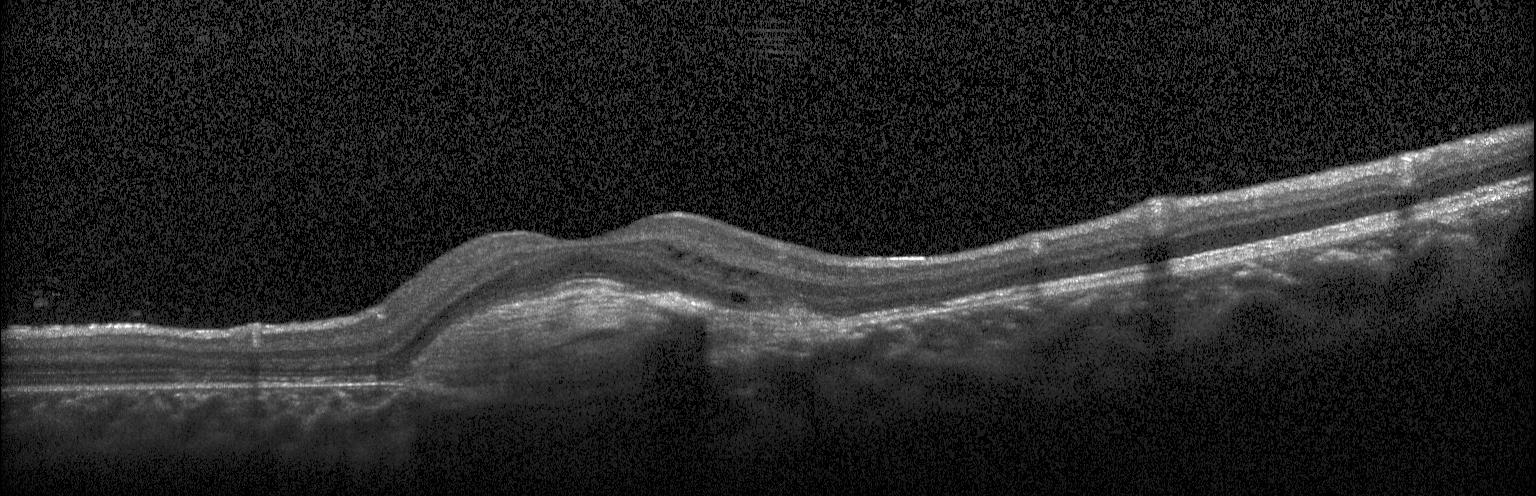
Optical coherence tomography B-scan.
Impression: CNV.